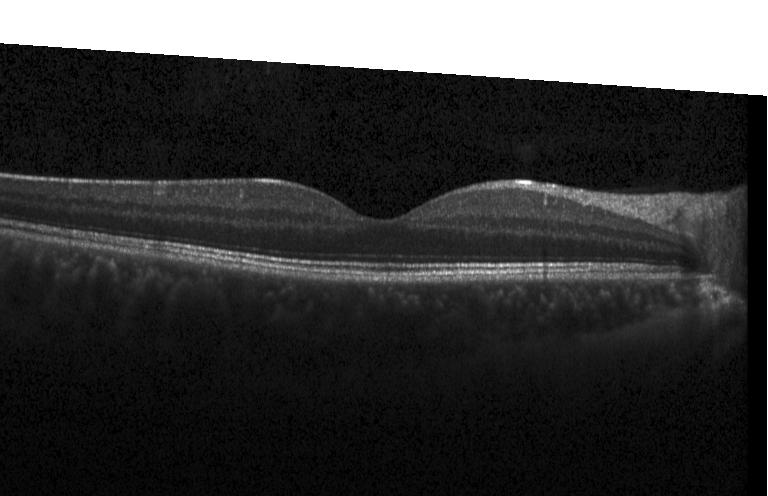
Optical coherence tomography scan
Finding: no CNV, DME, or drusen.